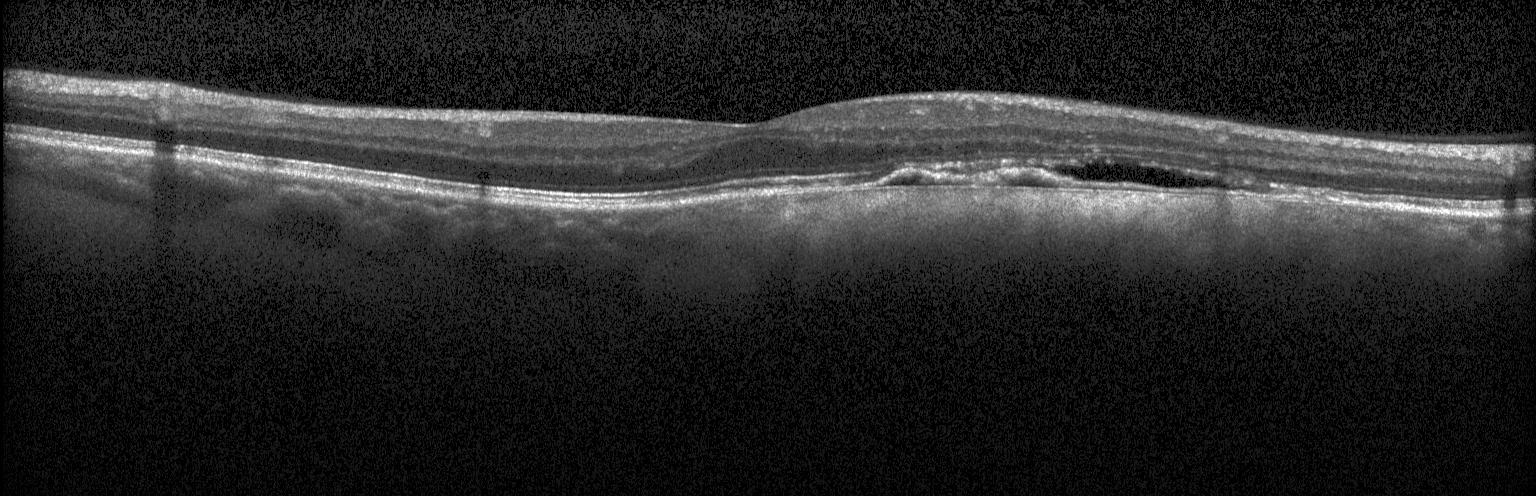
Diagnosis: a choroidal neovascular membrane.